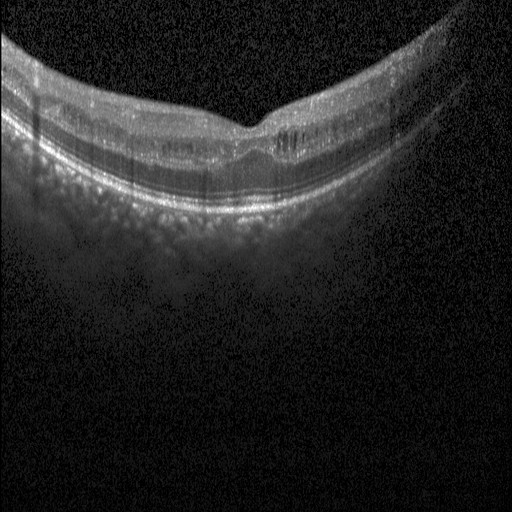

Heidelberg Spectralis OCT system; spectral-domain OCT; centered on the fovea; OCT B-scan. OCT finding: diabetic macular edema (DME).